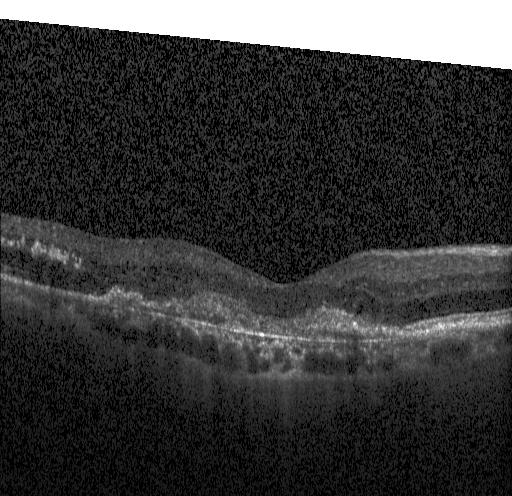
SD-OCT, optical coherence tomography B-scan, Heidelberg Spectralis — Impression: a choroidal neovascular membrane.